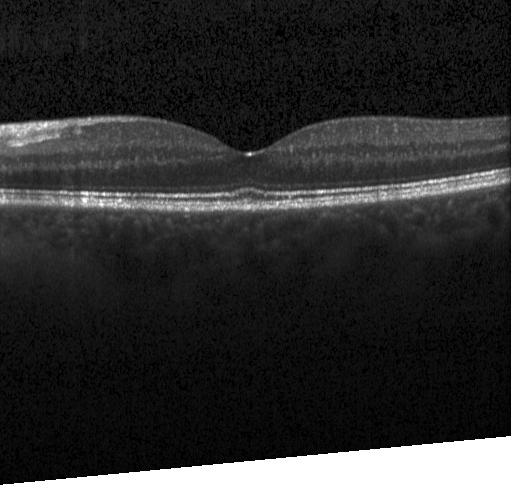 Horizontal scan through the fovea; spectral-domain OCT; acquired on a Heidelberg Spectralis; retinal OCT cross-section — No choroidal neovascularization, diabetic macular edema, or drusen.